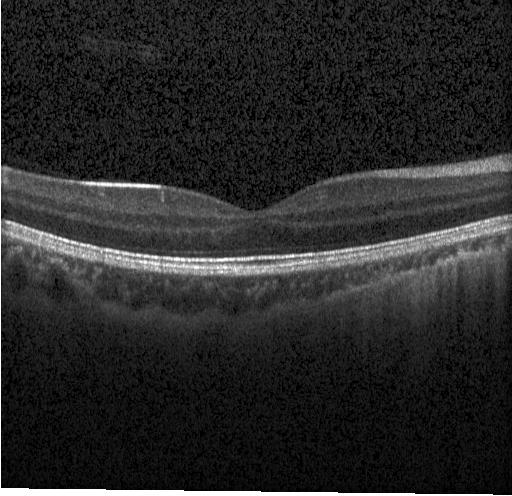
Diagnosis: no CNV, DME, or drusen.